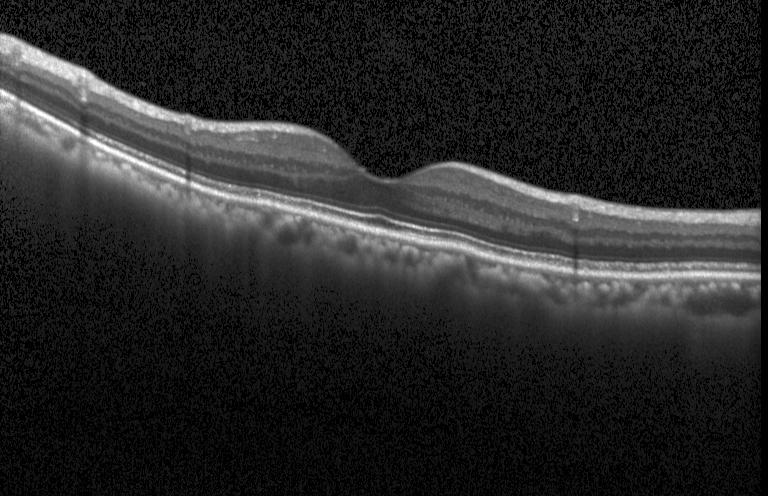
Finding: neither choroidal neovascularization, diabetic macular edema, nor drusen.